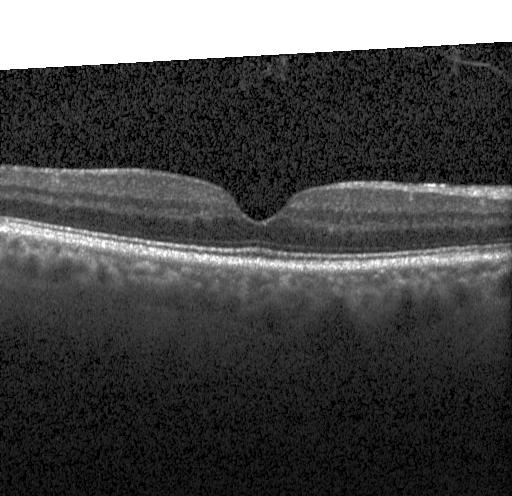
OCT B-scan · instrument: Heidelberg Spectralis · SD-OCT · through the macula — This B-scan demonstrates no CNV, DME, or drusen.